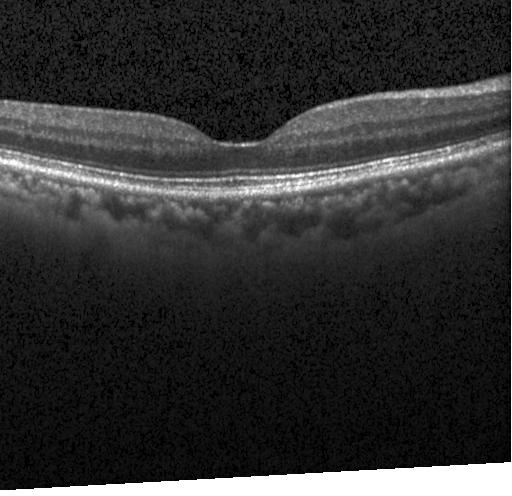

Finding: no choroidal neovascularization, diabetic macular edema, or drusen.